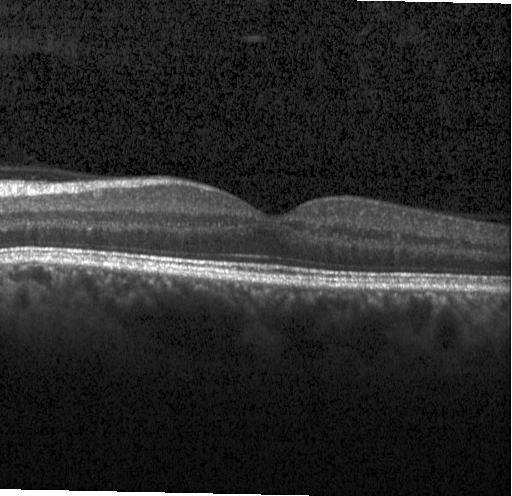 Instrument: Heidelberg Spectralis · macular scan · OCT line scan · spectral-domain optical coherence tomography
Impression: no evidence of choroidal neovascularization, diabetic macular edema, or drusen.